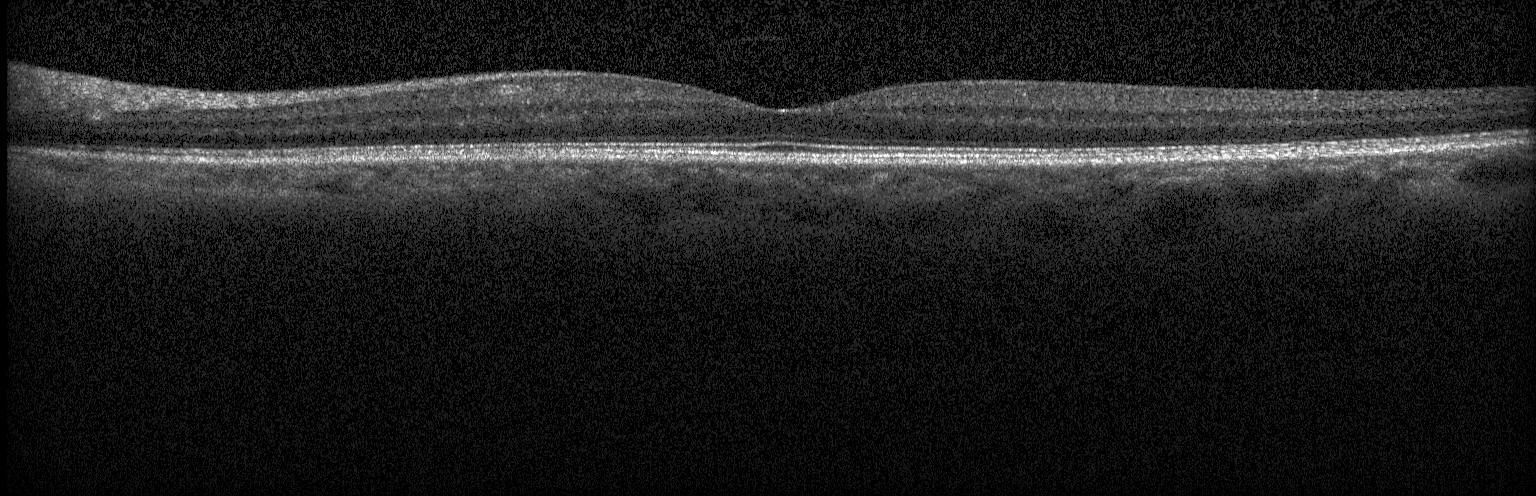 Retinal OCT B-scan
Dx: no choroidal neovascularization, no diabetic macular edema, and no drusen.